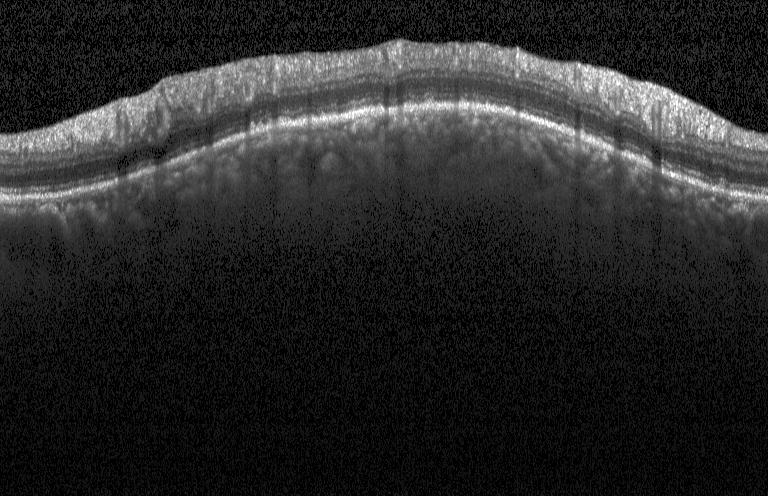
OCT B-scan.
This B-scan demonstrates CNV.